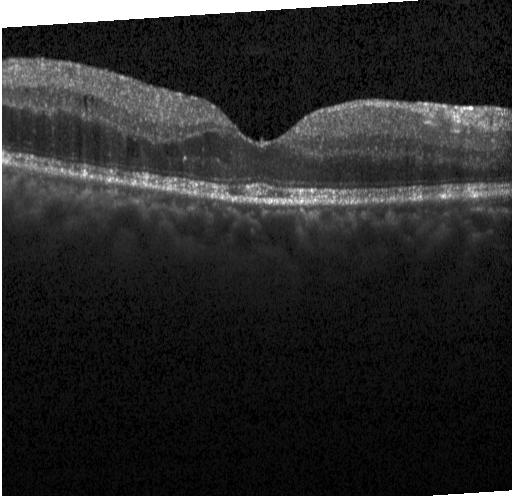
Optical coherence tomography B-scan — Dx: DME.